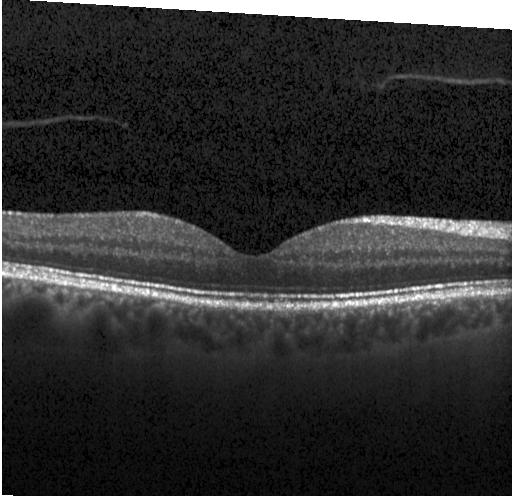
Acquired on a Heidelberg Spectralis; macular scan; spectral-domain OCT; retinal OCT cross-section
OCT finding: no evidence of CNV, DME, or drusen.